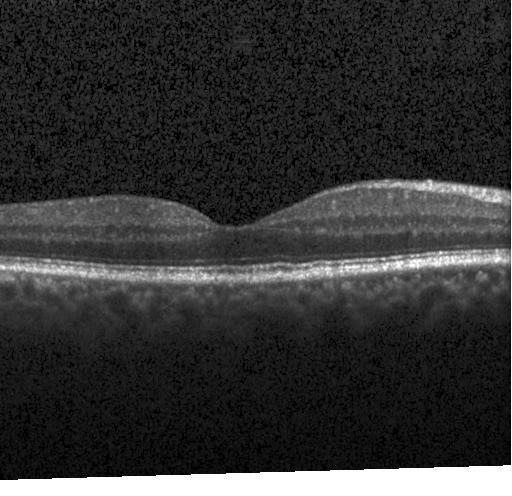
Heidelberg Spectralis OCT system. OCT line scan. Spectral-domain optical coherence tomography. Macular scan. Diagnosis: no evidence of CNV, DME, or drusen.